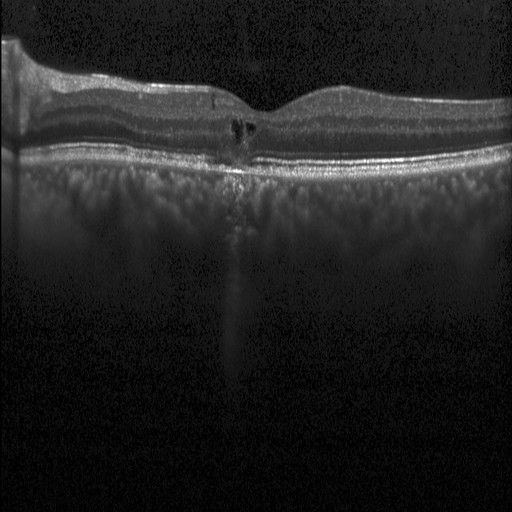 OCT scan showing diabetic macular edema (DME).